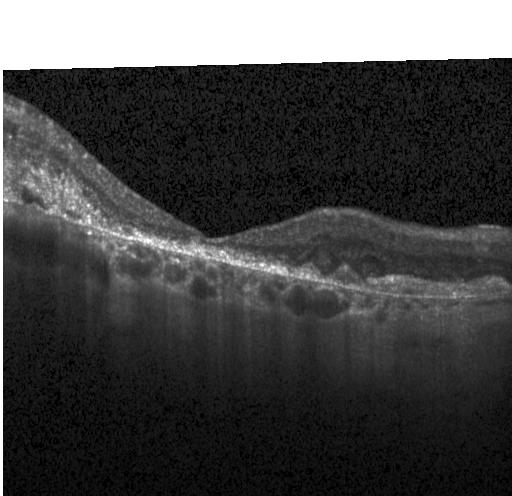

Horizontal scan through the fovea; optical coherence tomography scan; instrument: Heidelberg Spectralis. OCT finding: choroidal neovascularization (CNV).